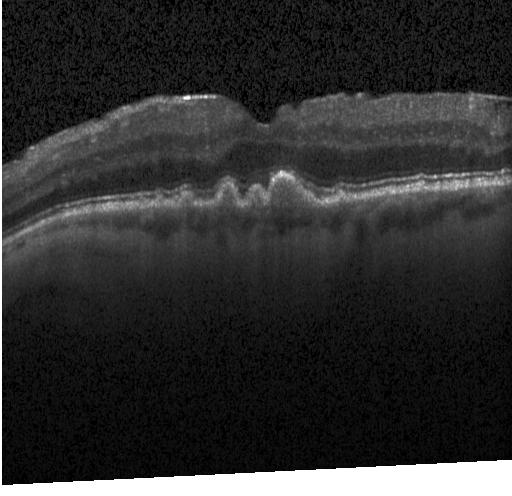
Spectral-domain OCT; optical coherence tomography scan — Diagnosis: drusen.